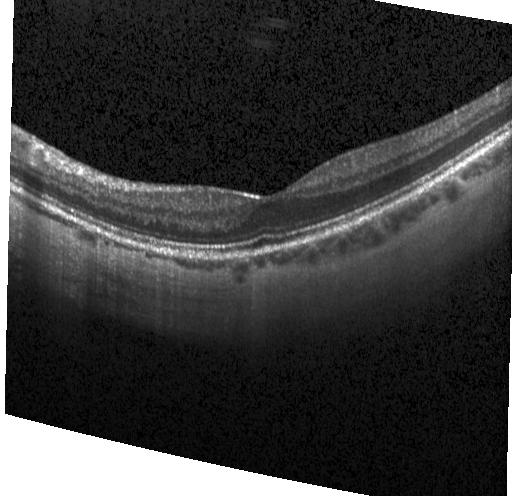

OCT line scan. The scan shows no evidence of CNV, DME, or drusen.